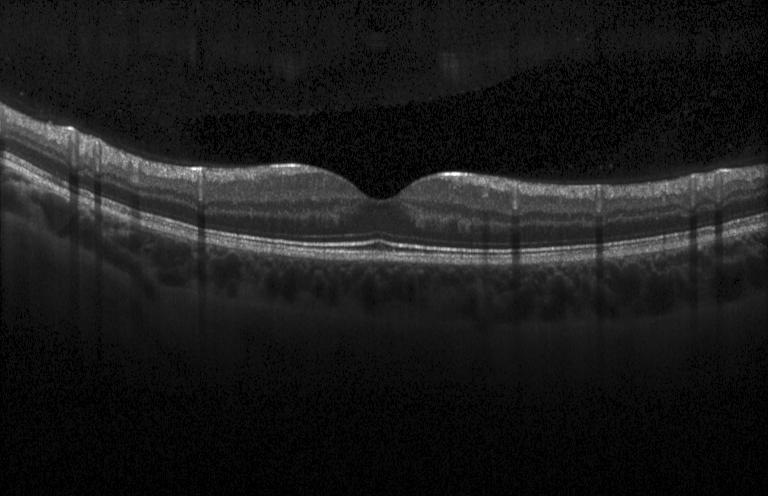 SD-OCT. Optical coherence tomography scan.
Assessment: no choroidal neovascularization, diabetic macular edema, or drusen.